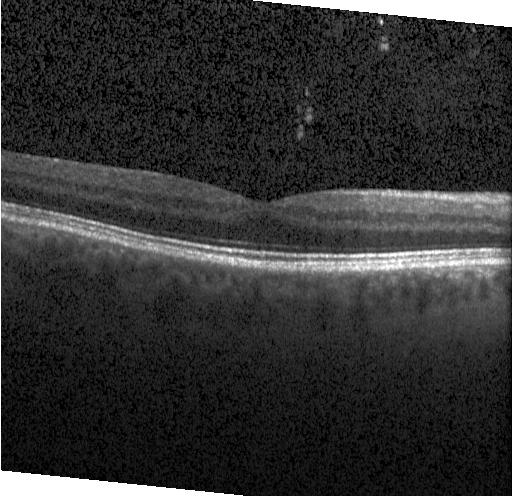
Finding: no choroidal neovascularization, diabetic macular edema, or drusen.